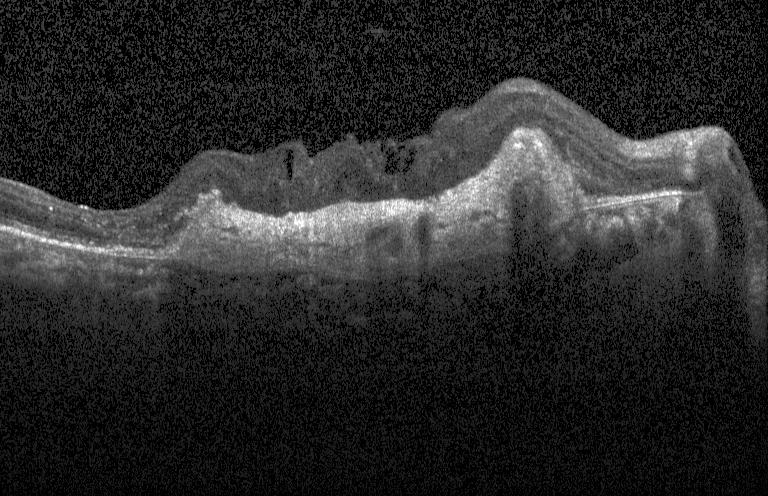

OCT line scan. Finding: a choroidal neovascular membrane.